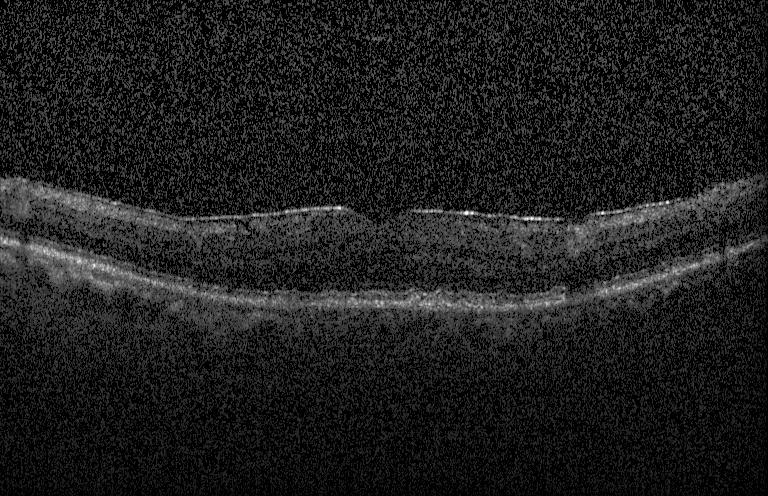
Diagnosis: sub-RPE drusenoid deposits.